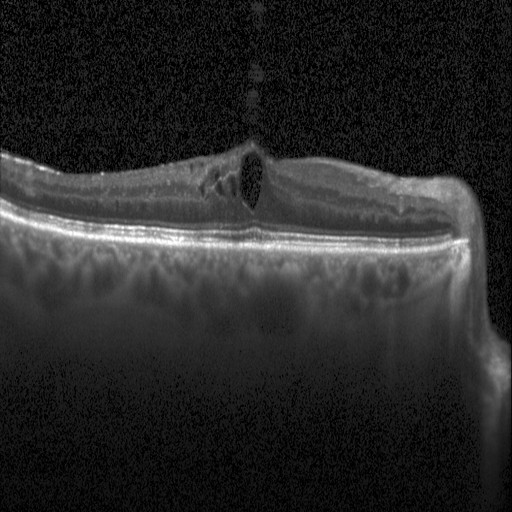 Heidelberg Spectralis. Optical coherence tomography B-scan — Diagnosis: diabetic macular edema.